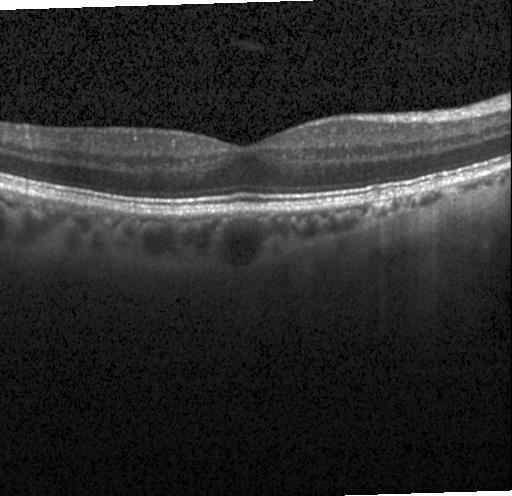
Optical coherence tomography B-scan; centered on the fovea.
Impression: no evidence of choroidal neovascularization, diabetic macular edema, or drusen.